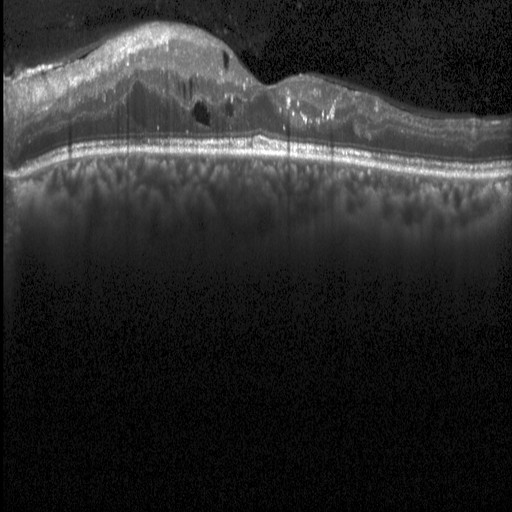

Macular OCT: diabetic macular edema (DME).